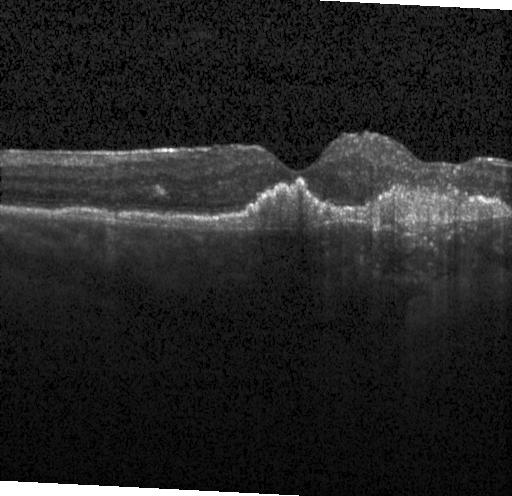
Heidelberg Spectralis. Spectral-domain OCT. Centered on the fovea. Optical coherence tomography scan.
Dx: a choroidal neovascular membrane.